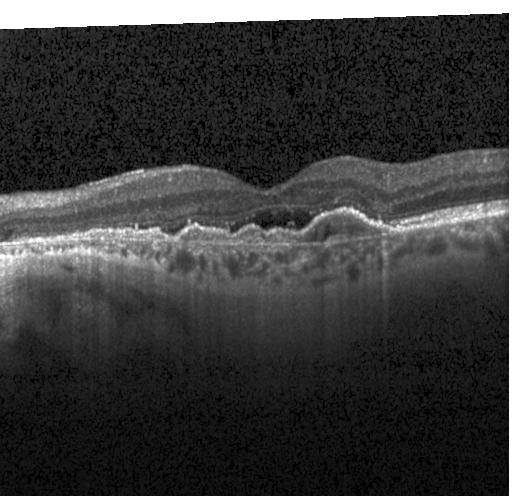 Impression: choroidal neovascularization.